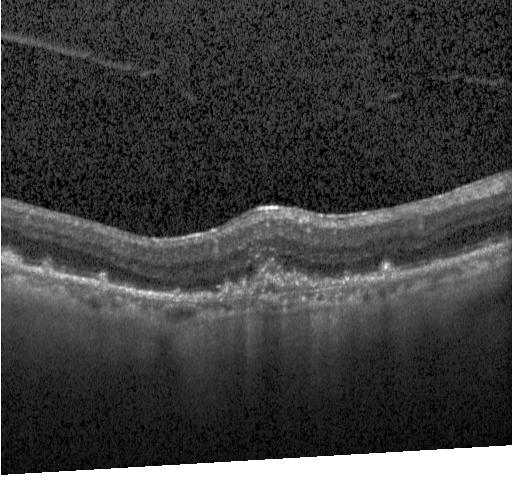 OCT scan showing choroidal neovascularization (CNV).